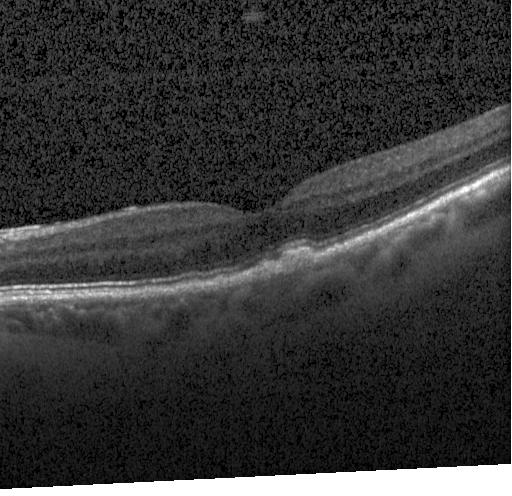
Retinal OCT B-scan
Finding: multiple drusen.